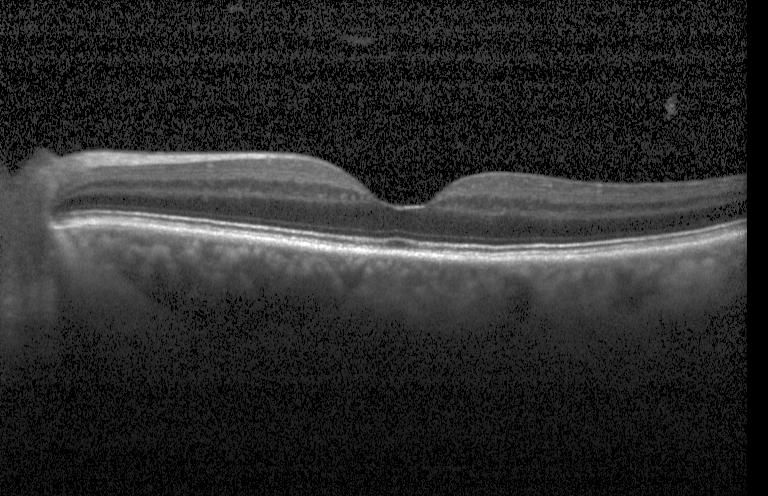
Heidelberg Spectralis OCT system, retinal OCT B-scan, spectral-domain optical coherence tomography. Diagnosis: no choroidal neovascularization, diabetic macular edema, or drusen.